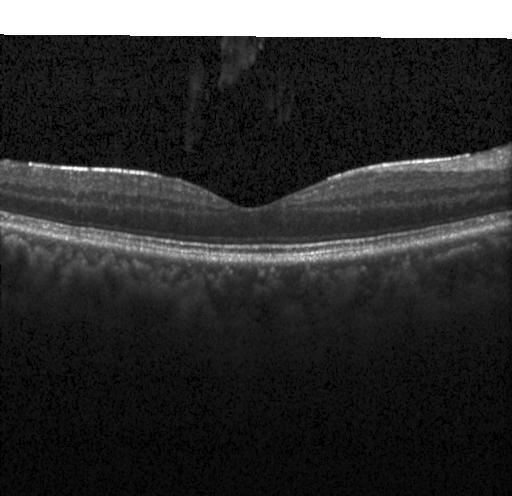
Macular OCT: no choroidal neovascularization, no diabetic macular edema, and no drusen.